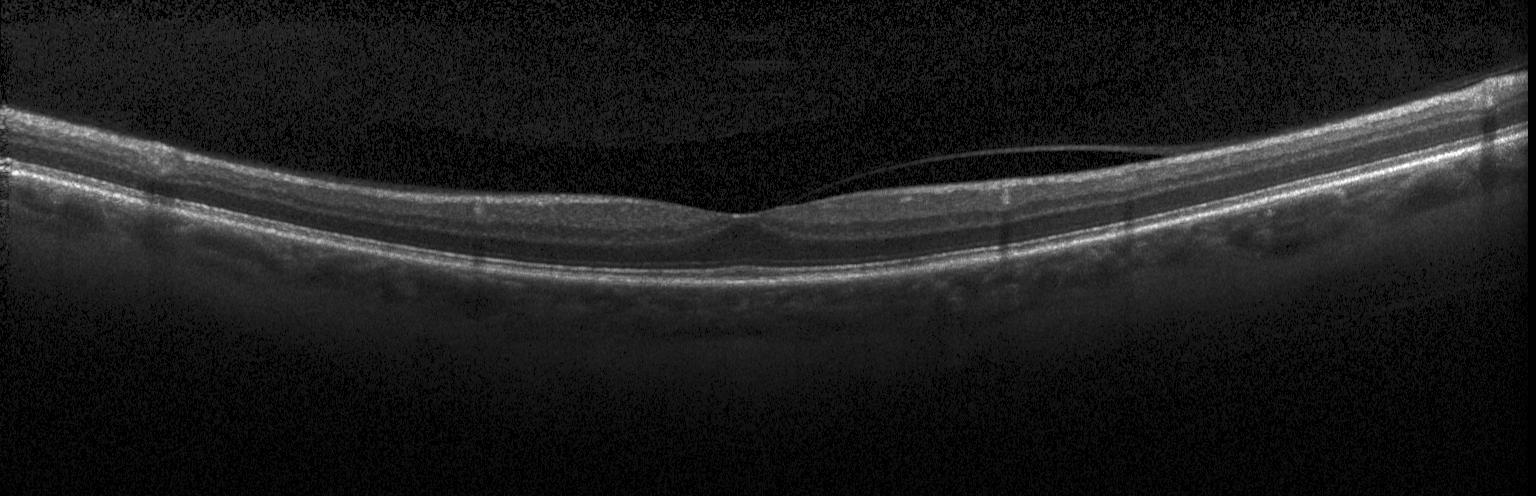 Retinal OCT cross-section · instrument: Heidelberg Spectralis · spectral-domain OCT · through the macula. Finding: no choroidal neovascularization, diabetic macular edema, or drusen.